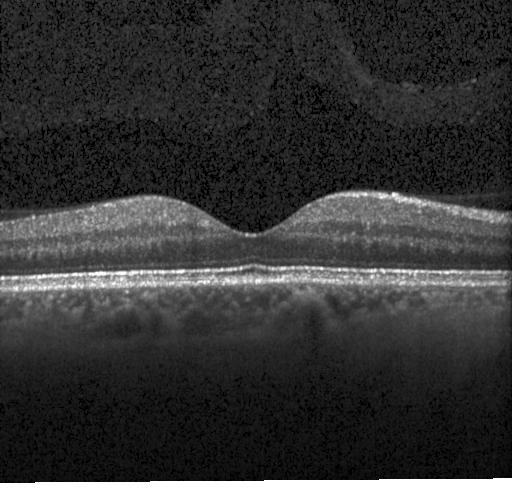 Spectral-domain optical coherence tomography. Heidelberg Spectralis OCT system. Retinal OCT cross-section
Neither choroidal neovascularization, diabetic macular edema, nor drusen.